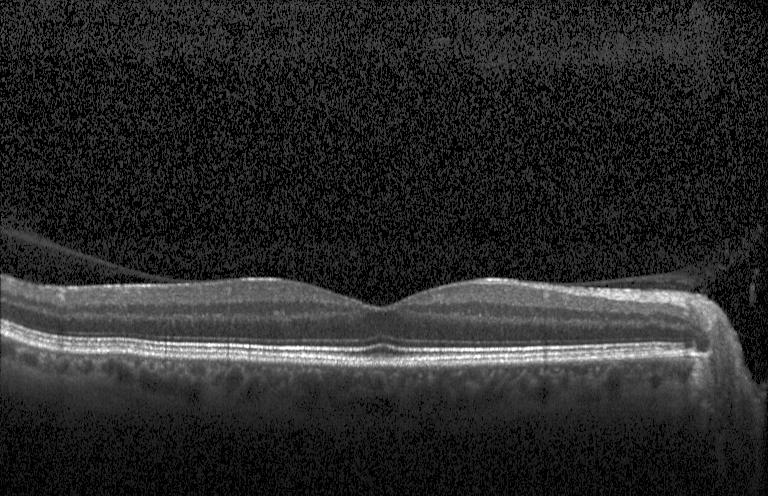 Diagnosis: no choroidal neovascularization, no diabetic macular edema, and no drusen.